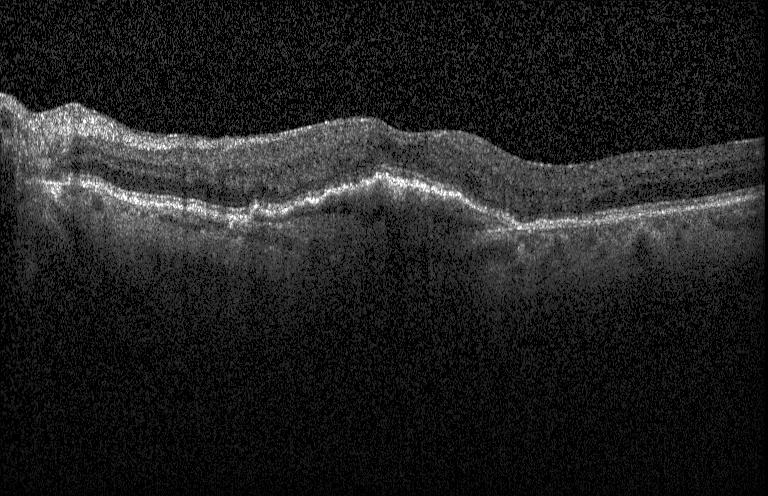

Macular OCT: choroidal neovascularization.